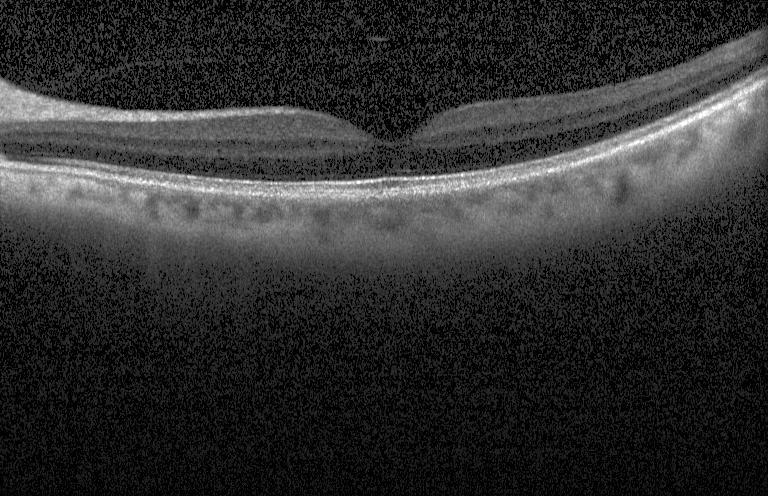 OCT B-scan showing no evidence of choroidal neovascularization, diabetic macular edema, or drusen.